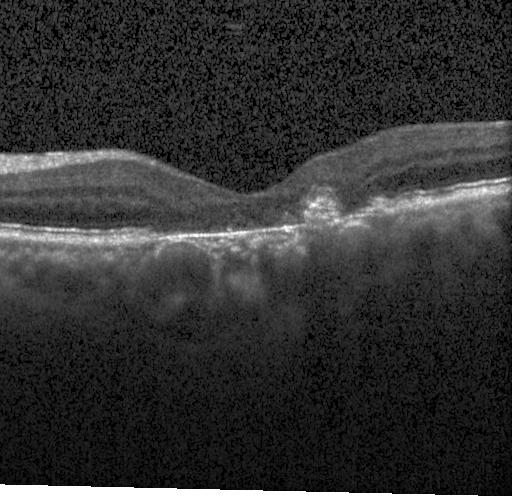

Retinal OCT B-scan. Acquired on a Heidelberg Spectralis.
The scan shows a choroidal neovascular membrane.